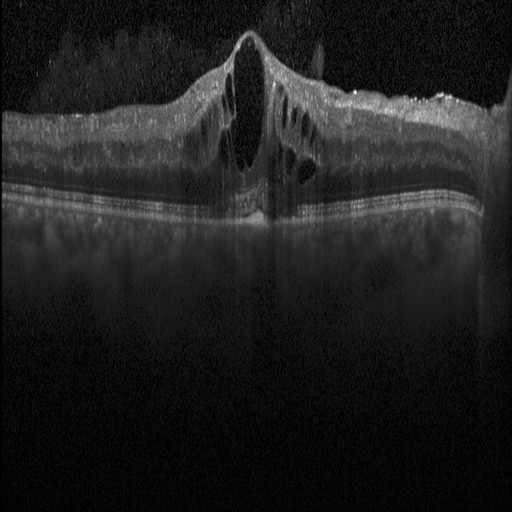
OCT B-scan; acquired on a Heidelberg Spectralis; spectral-domain optical coherence tomography; centered on the fovea — Impression: DME.